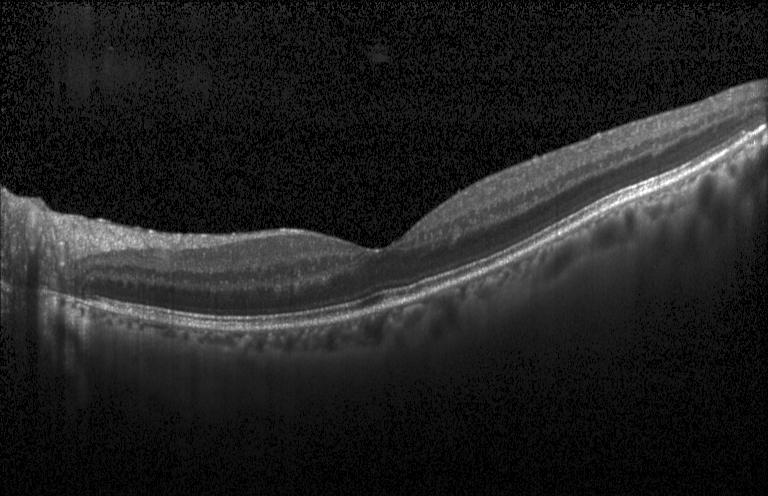

Retinal OCT B-scan. Dx: neither CNV, DME, nor drusen.